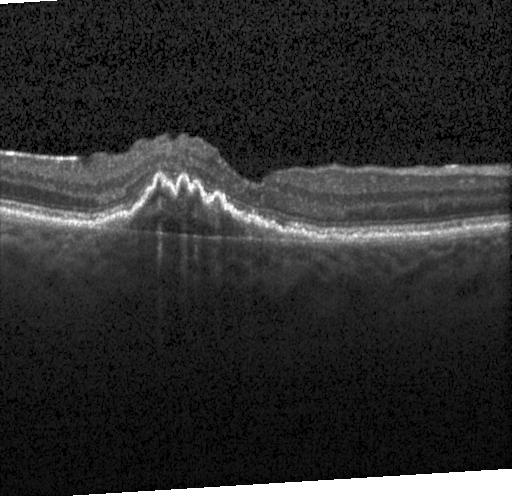
OCT scan showing choroidal neovascularization.